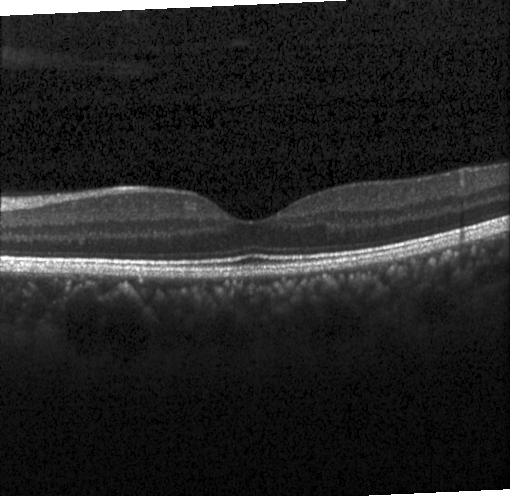

Through the macula; OCT B-scan; Heidelberg Spectralis; spectral-domain optical coherence tomography
This B-scan demonstrates no choroidal neovascularization, diabetic macular edema, or drusen.